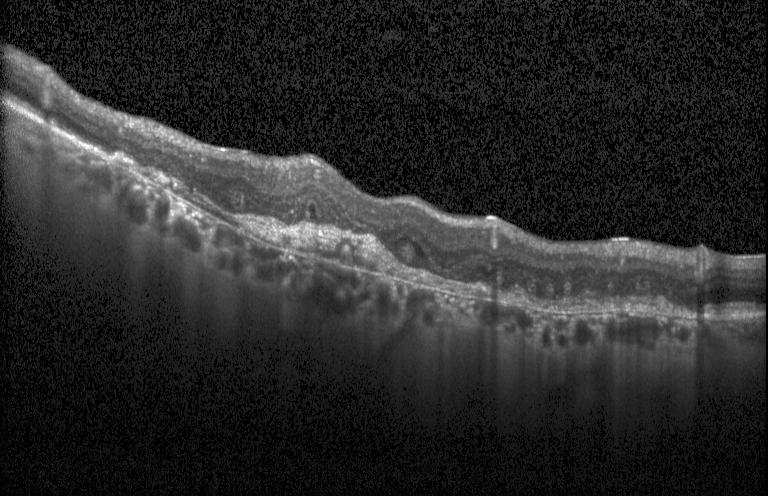

Retinal OCT B-scan · horizontal scan through the fovea · SD-OCT
Diagnosis: a choroidal neovascular membrane.